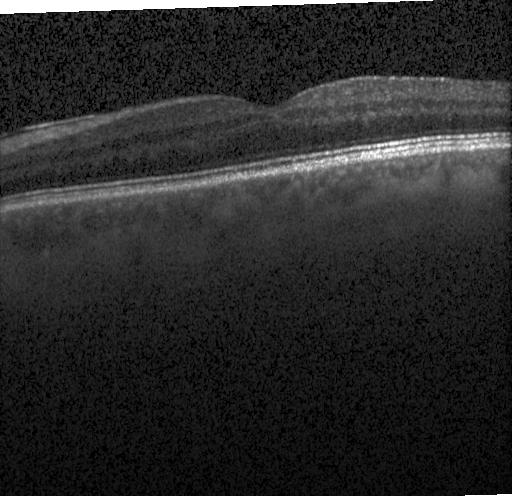 Retinal OCT cross-section
Assessment: neither CNV, DME, nor drusen.